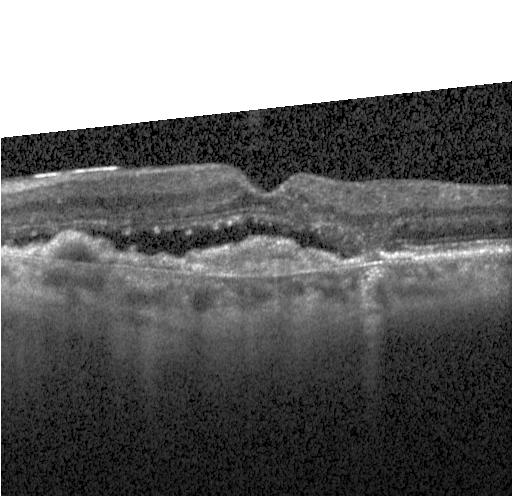
Macular OCT: a choroidal neovascular membrane.